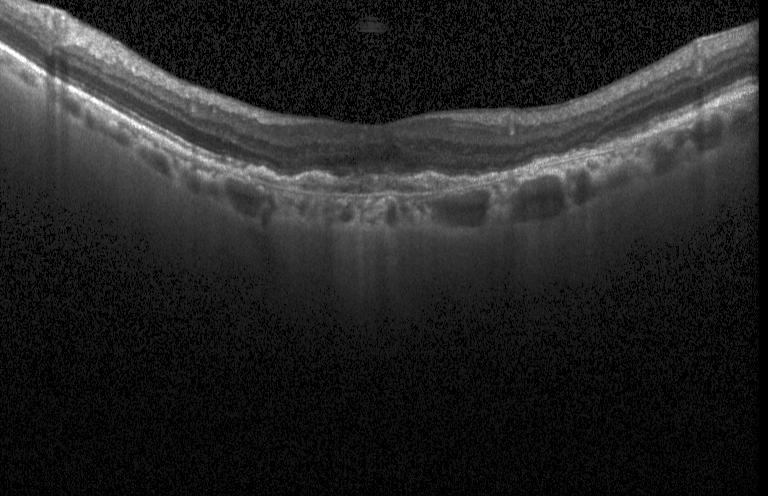
OCT finding: a choroidal neovascular membrane.